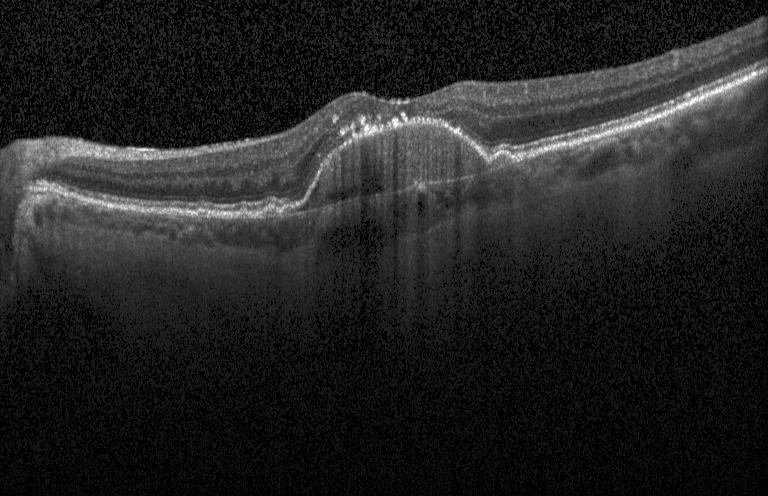 Macular scan · optical coherence tomography B-scan.
Impression: CNV.